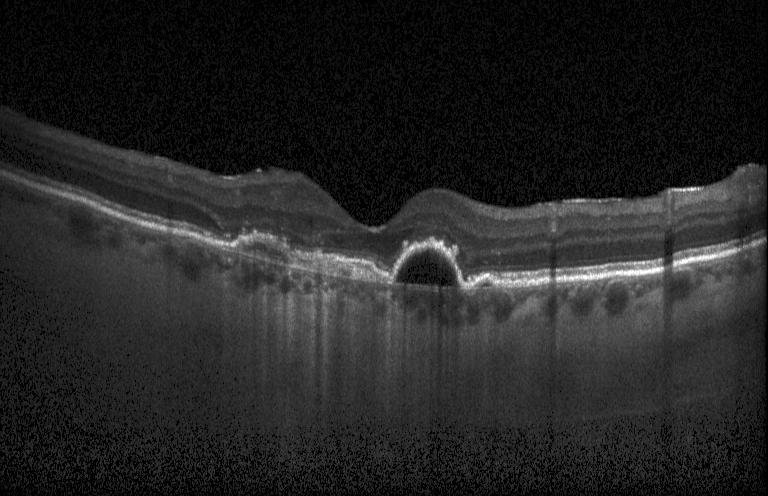

Macular OCT: a choroidal neovascular membrane.